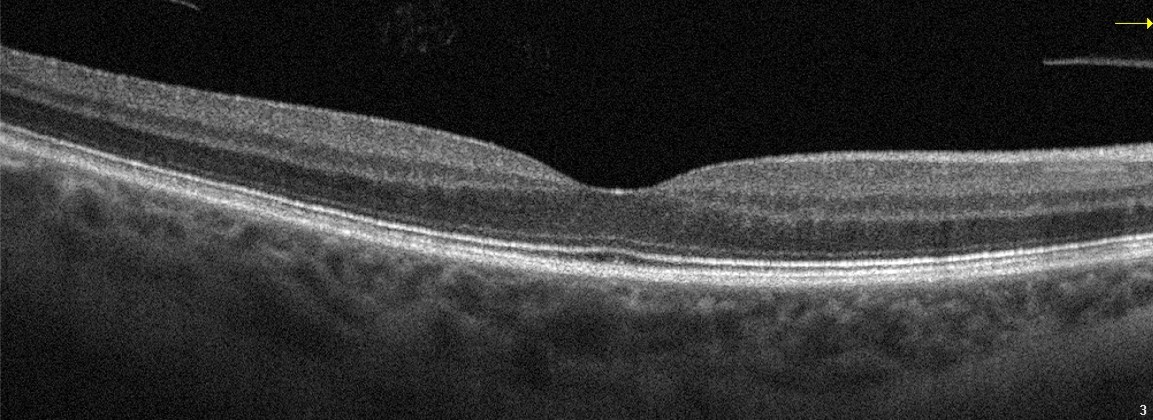

Diagnosis: absence of AMD, DME, ERM, RAO, RVO, and vitreomacular interface disease.